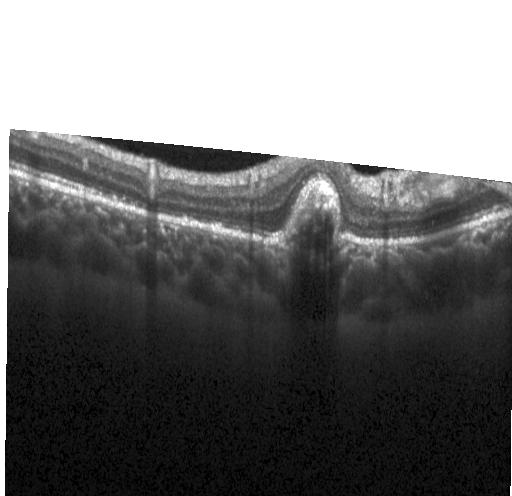

Impression: a choroidal neovascular membrane.